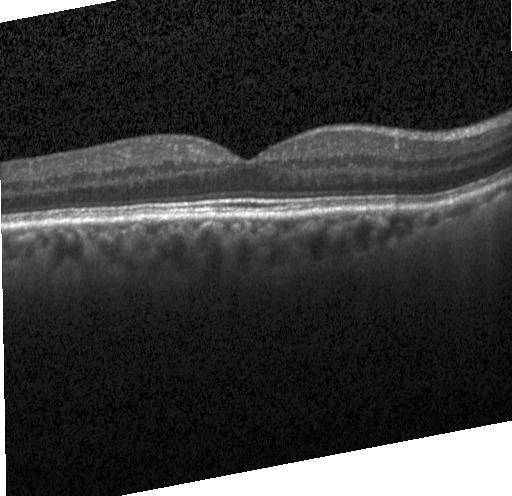
Retinal OCT cross-section showing no choroidal neovascularization, no diabetic macular edema, and no drusen.